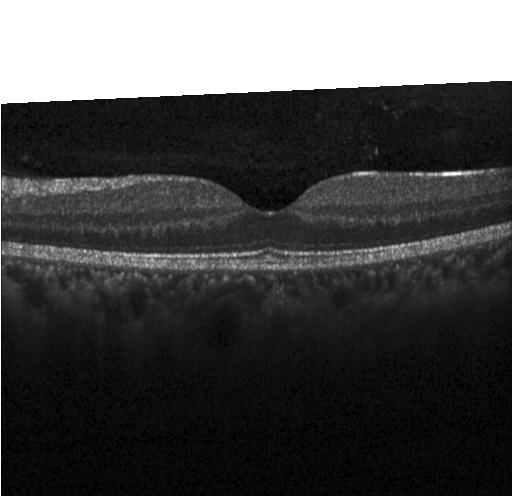 Retinal OCT cross-section · instrument: Heidelberg Spectralis. Macular OCT: no evidence of choroidal neovascularization, diabetic macular edema, or drusen.